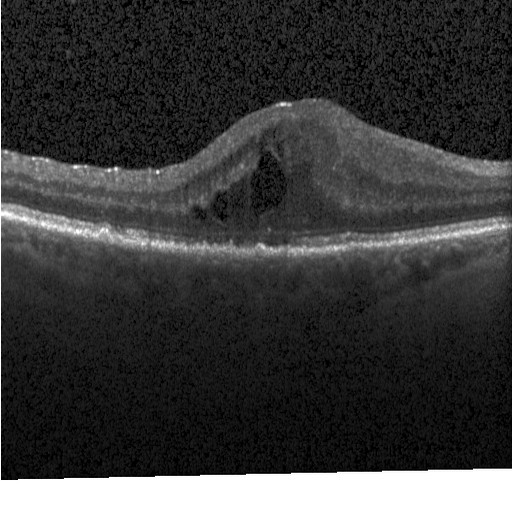

OCT B-scan showing diabetic macular edema (DME).